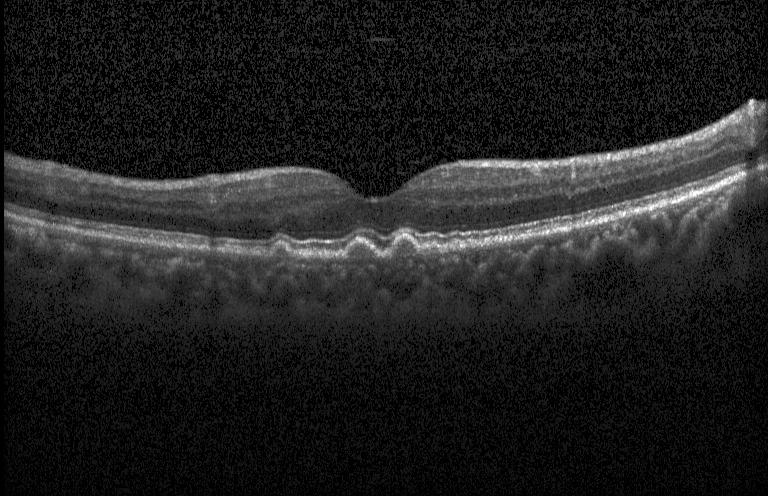

Heidelberg Spectralis. Fovea-centered. SD-OCT. Retinal OCT B-scan.
Impression: multiple drusen.